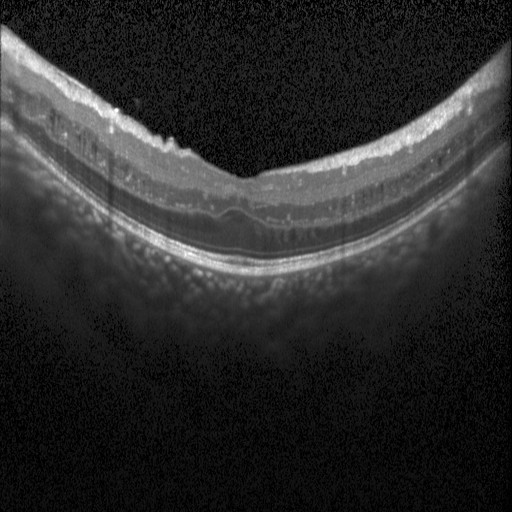
OCT finding: DME.